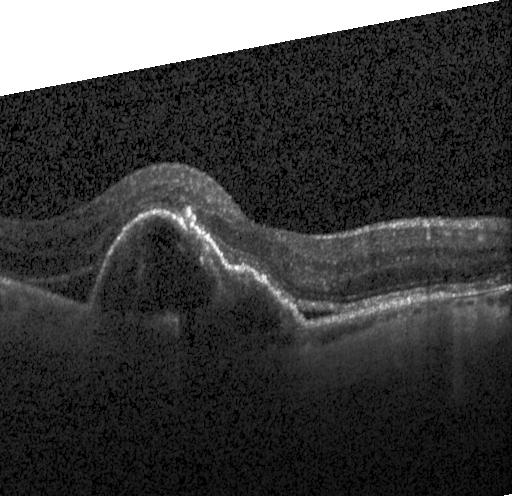
Diagnosis: a choroidal neovascular membrane.